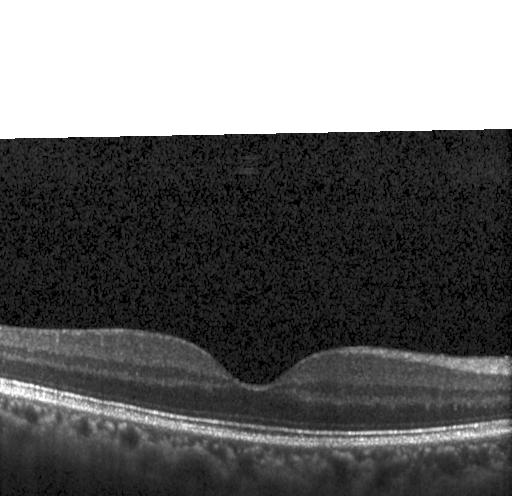 OCT line scan
Impression: no choroidal neovascularization, no diabetic macular edema, and no drusen.